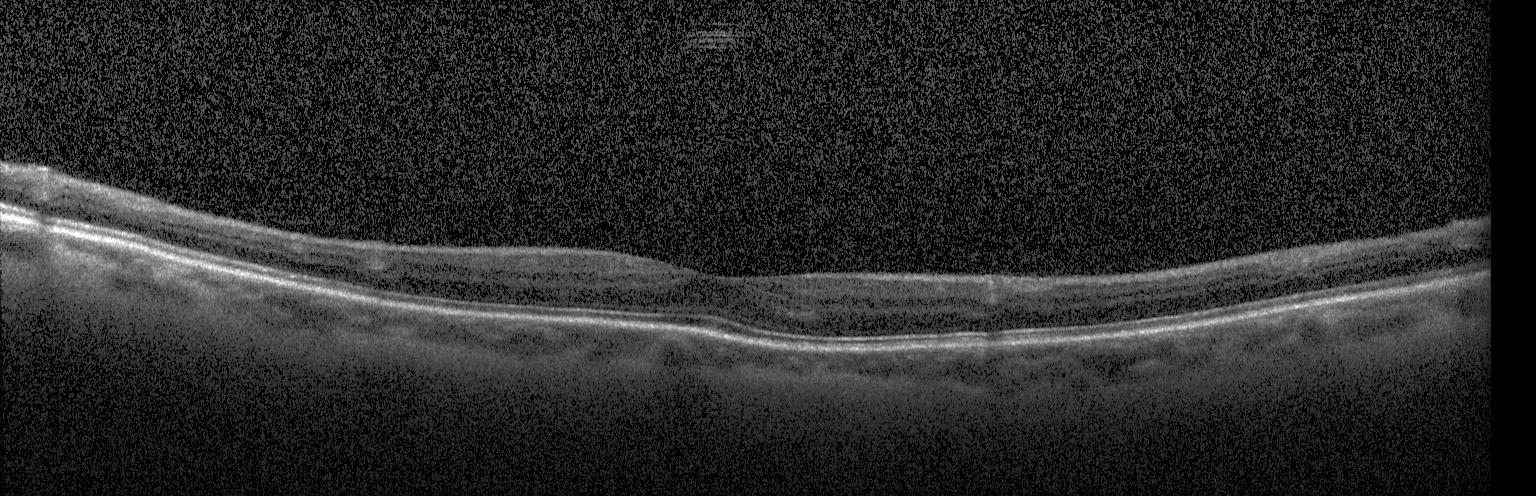

OCT line scan, acquired on a Heidelberg Spectralis.
This B-scan demonstrates no choroidal neovascularization, diabetic macular edema, or drusen.